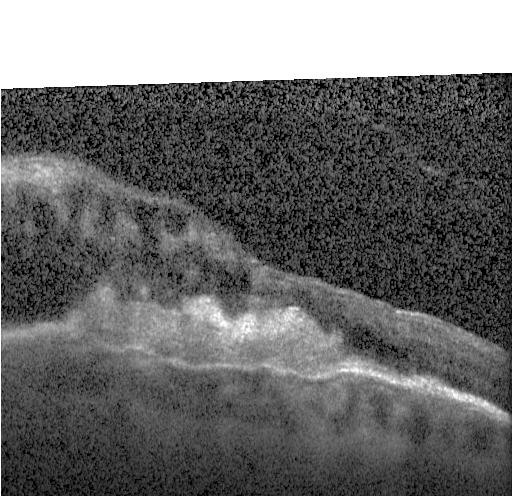
Spectral-domain OCT, through the macula, acquired on a Heidelberg Spectralis, OCT B-scan — Macular OCT: a choroidal neovascular membrane.